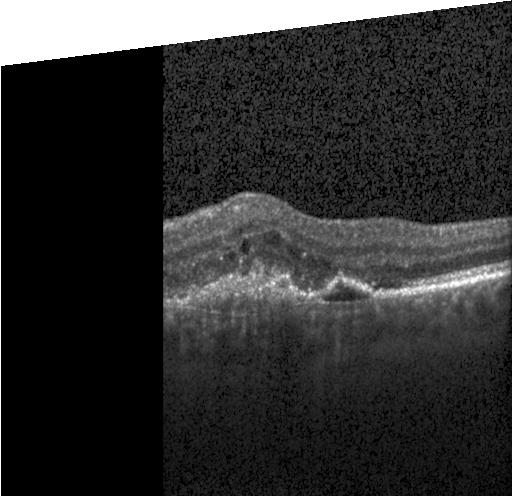 Optical coherence tomography scan, acquired on a Heidelberg Spectralis, horizontal scan through the fovea
This B-scan demonstrates choroidal neovascularization.